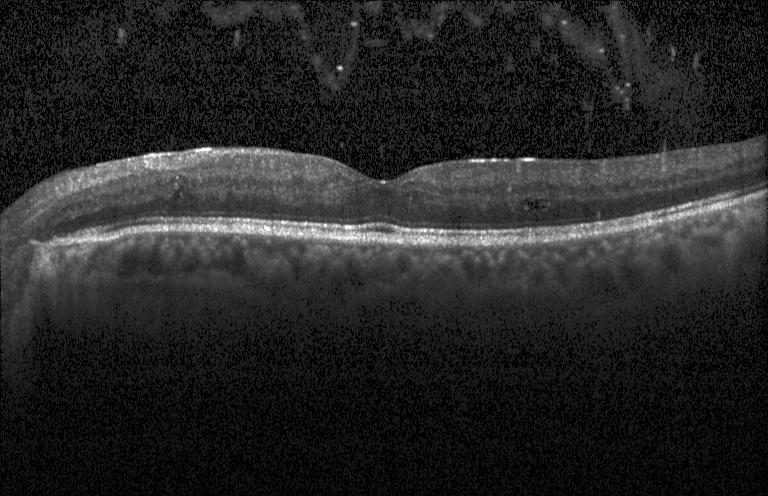
OCT finding: DME.